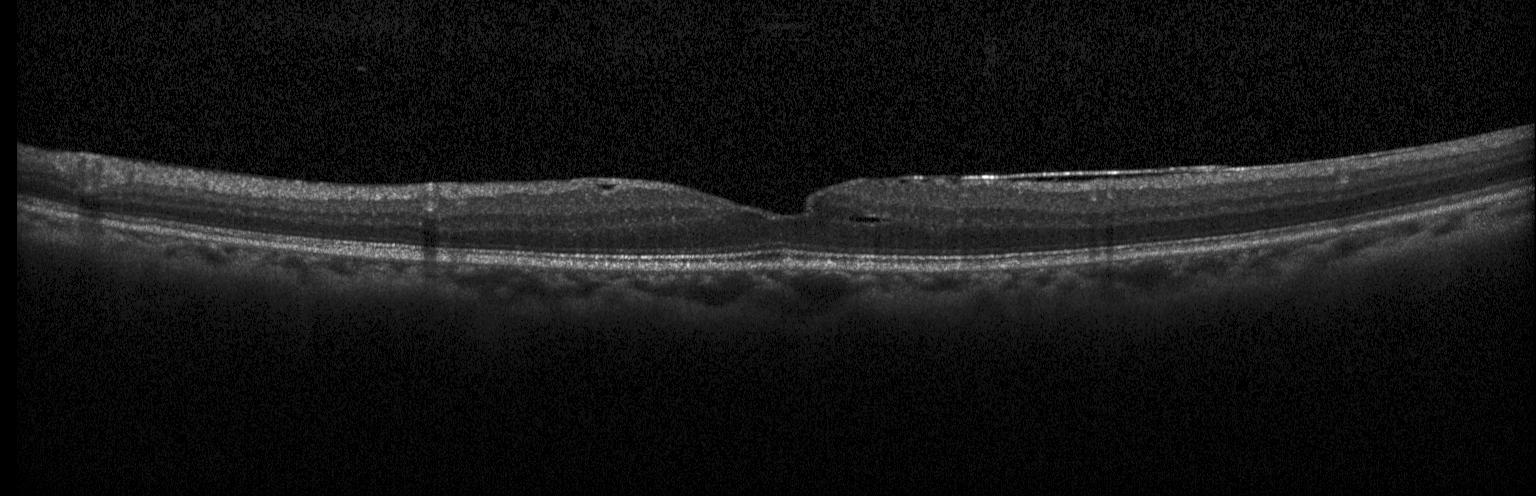

Impression: diabetic macular edema.